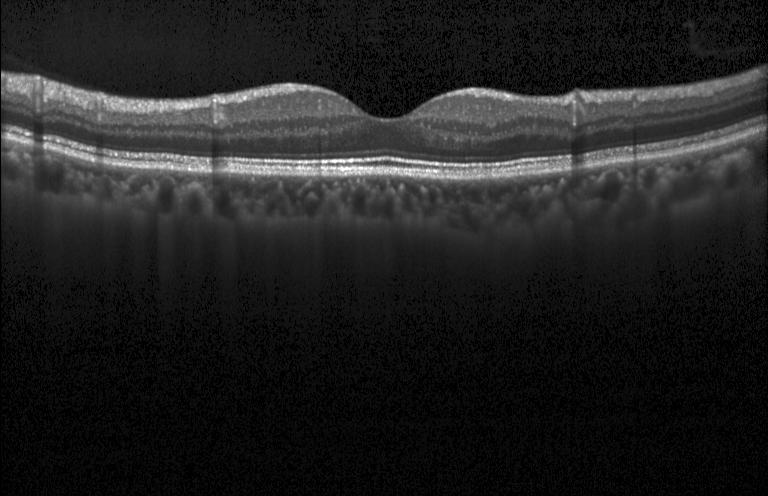 Optical coherence tomography B-scan
Assessment: no choroidal neovascularization, no diabetic macular edema, and no drusen.